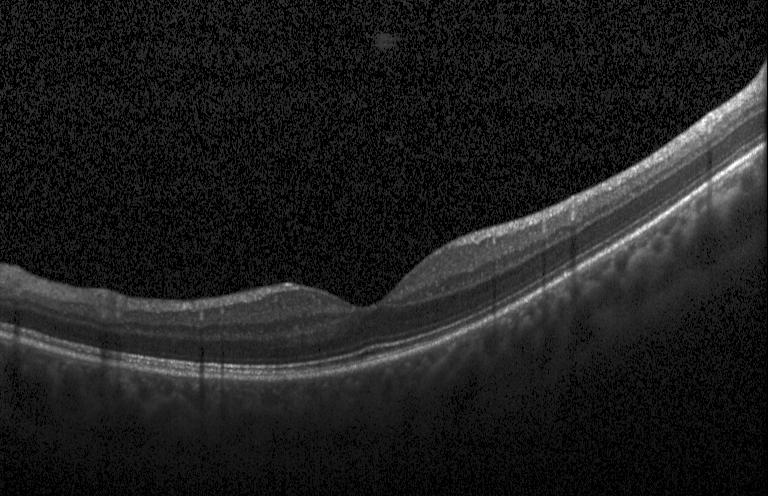
Heidelberg Spectralis, optical coherence tomography B-scan.
OCT finding: no CNV, DME, or drusen.